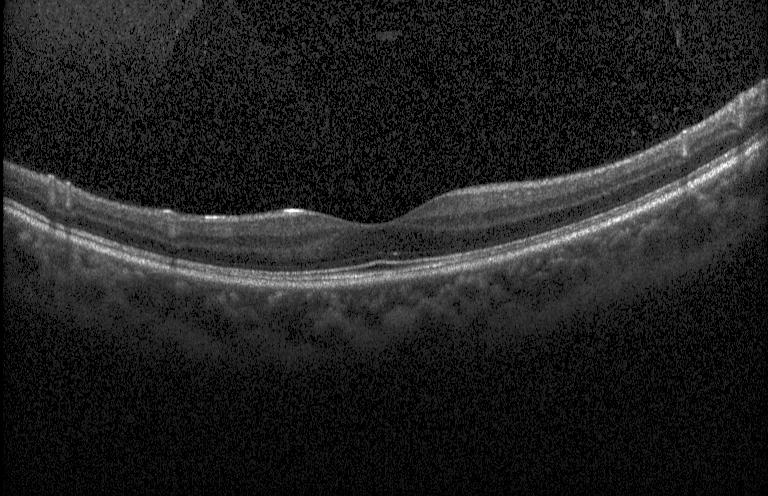 Retinal OCT cross-section · spectral-domain optical coherence tomography · instrument: Heidelberg Spectralis.
Finding: no evidence of choroidal neovascularization, diabetic macular edema, or drusen.